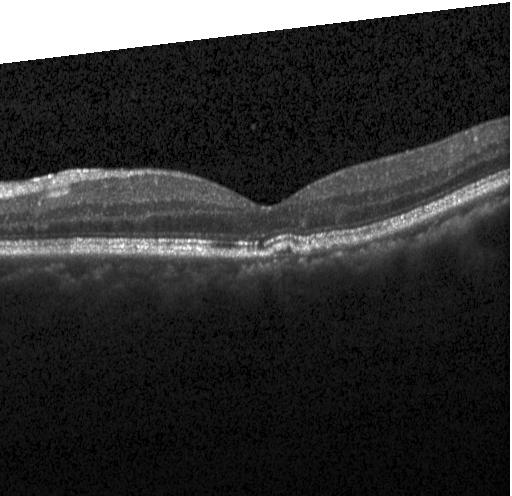 Heidelberg Spectralis; optical coherence tomography B-scan — The scan shows sub-RPE drusenoid deposits.